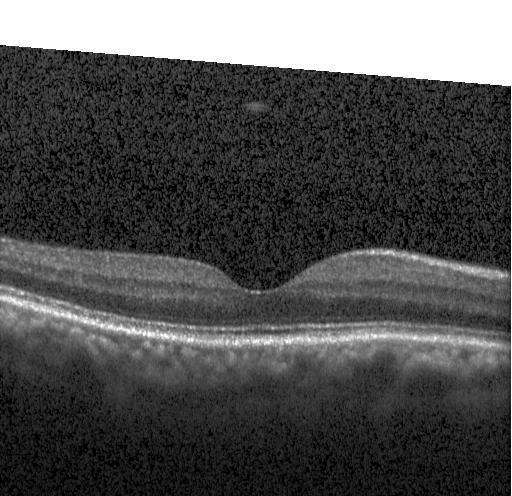

Spectral-domain optical coherence tomography; instrument: Heidelberg Spectralis; retinal OCT cross-section.
No choroidal neovascularization, no diabetic macular edema, and no drusen.